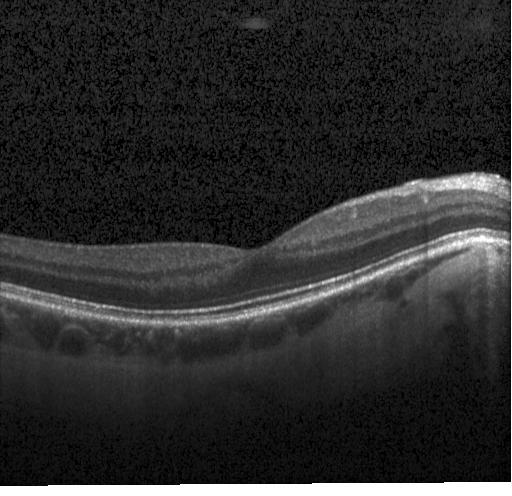

Heidelberg Spectralis OCT system · optical coherence tomography scan · spectral-domain optical coherence tomography · fovea-centered.
Dx: no evidence of CNV, DME, or drusen.